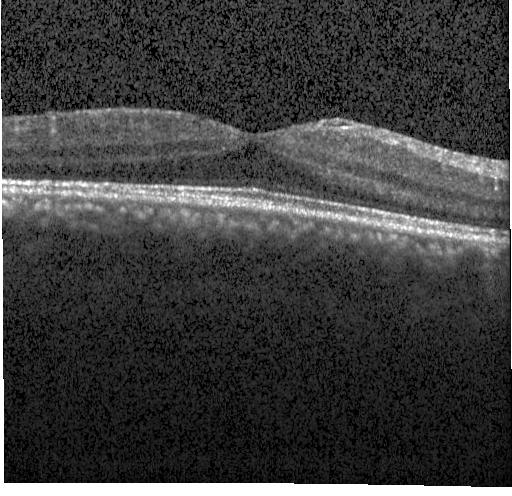
Retinal OCT B-scan.
Finding: no evidence of choroidal neovascularization, diabetic macular edema, or drusen.